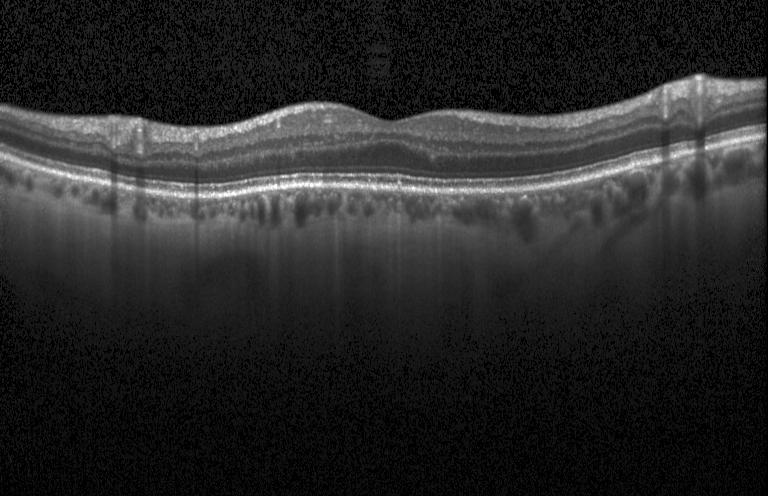
Through the macula, spectral-domain optical coherence tomography, optical coherence tomography B-scan, Heidelberg Spectralis OCT system
Impression: no evidence of CNV, DME, or drusen.